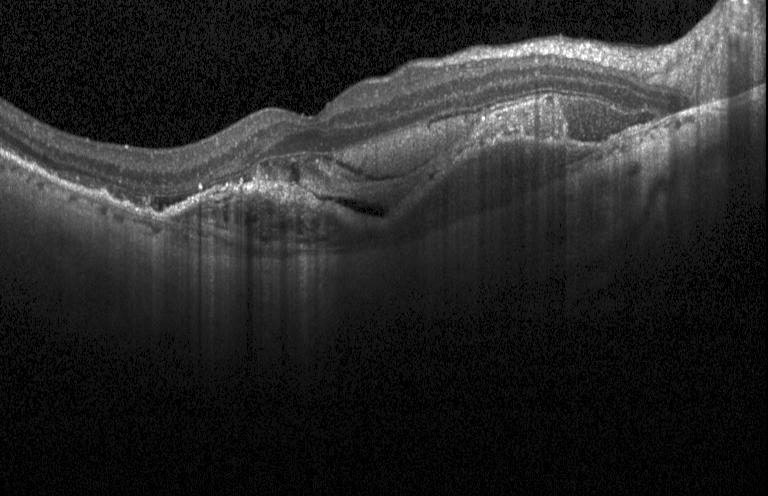 Macular OCT demonstrating choroidal neovascularization.